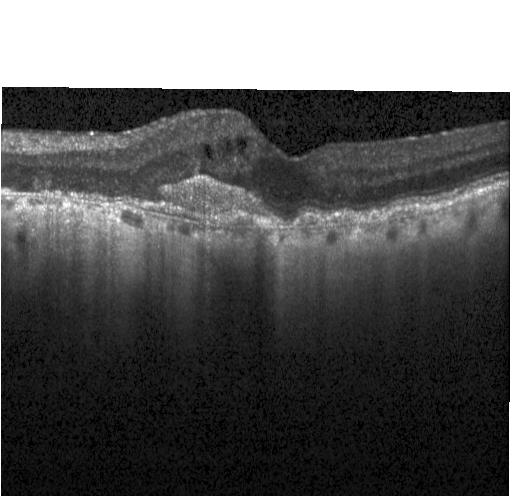

OCT B-scan · spectral-domain OCT · fovea-centered
Diagnosis: choroidal neovascularization.